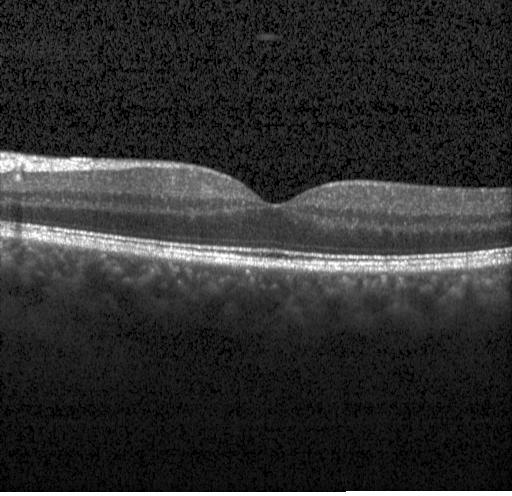

This B-scan demonstrates no evidence of choroidal neovascularization, diabetic macular edema, or drusen.